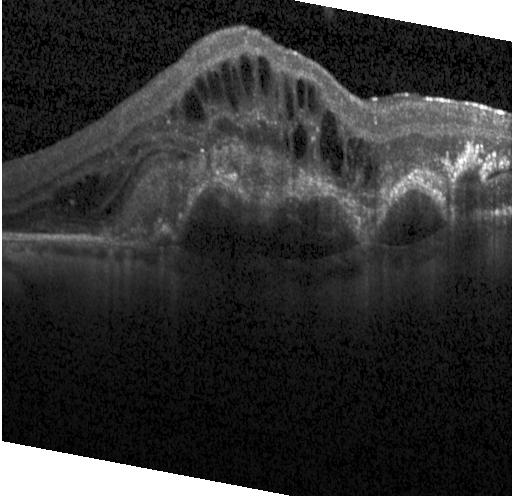 Optical coherence tomography scan, acquired on a Heidelberg Spectralis, macular scan. Macular OCT: CNV.